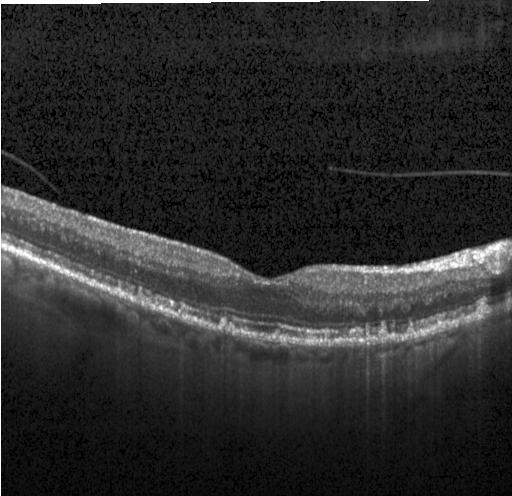 Finding: sub-RPE drusenoid deposits.